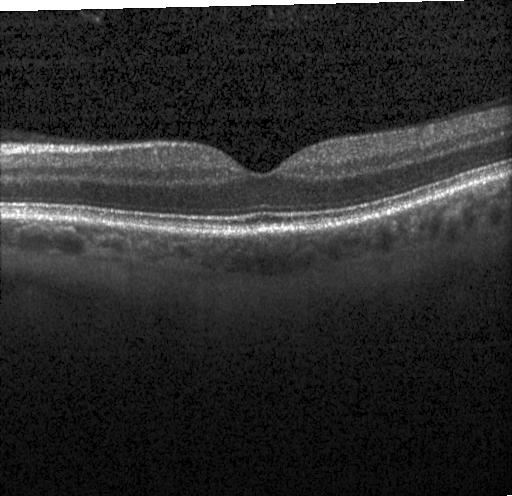 Through the macula. OCT B-scan. Finding: no evidence of choroidal neovascularization, diabetic macular edema, or drusen.